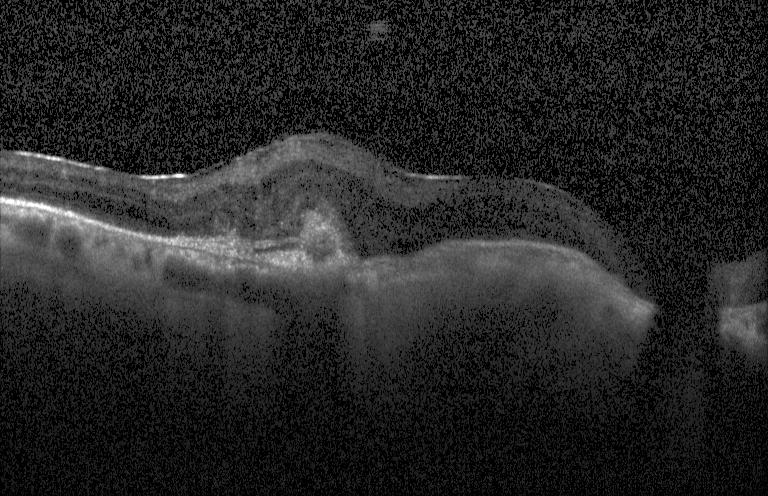 Dx: a choroidal neovascular membrane.